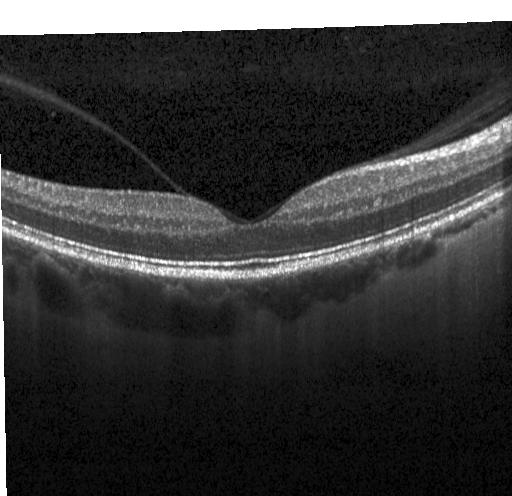

Impression: no choroidal neovascularization, diabetic macular edema, or drusen.